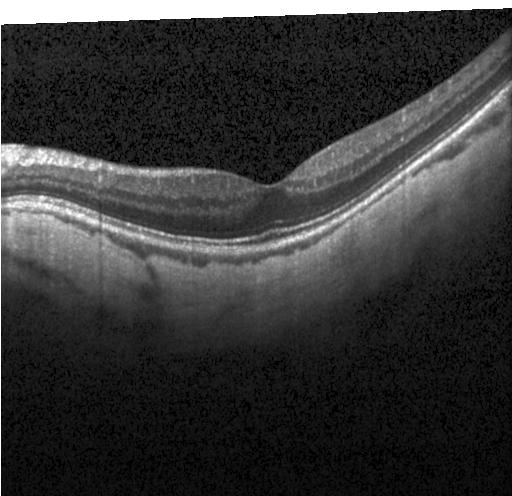

Macular OCT: no evidence of CNV, DME, or drusen.